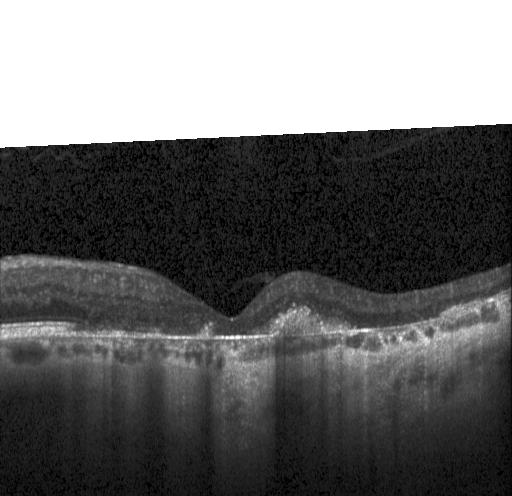 Retinal OCT B-scan, fovea-centered. This B-scan demonstrates a choroidal neovascular membrane.